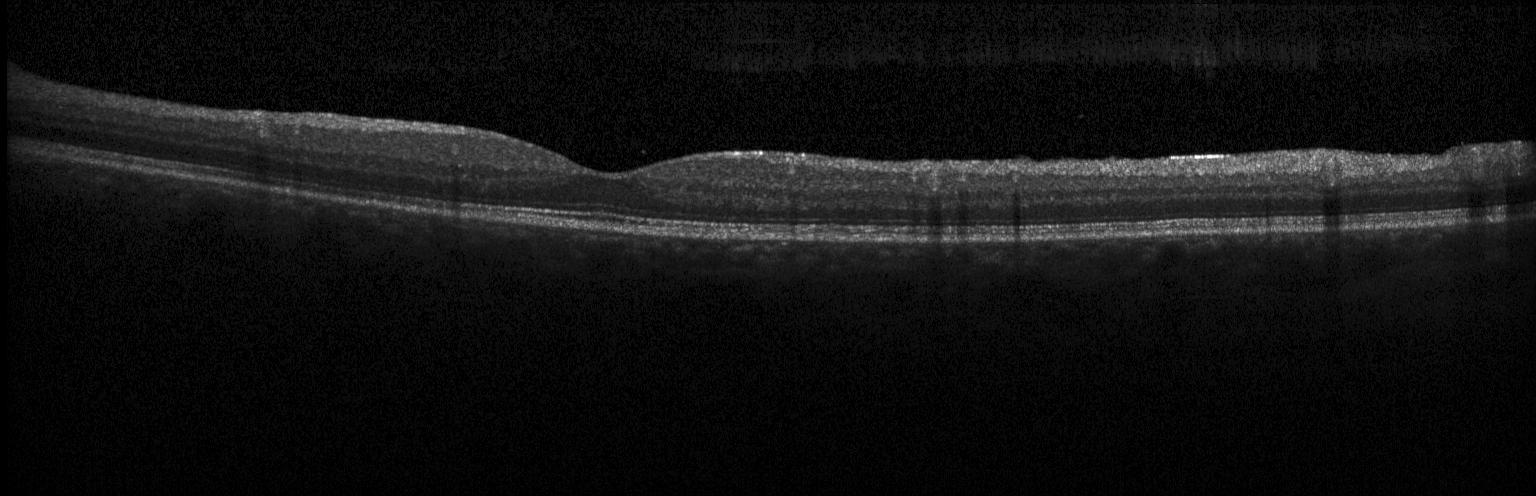
Neither choroidal neovascularization, diabetic macular edema, nor drusen.